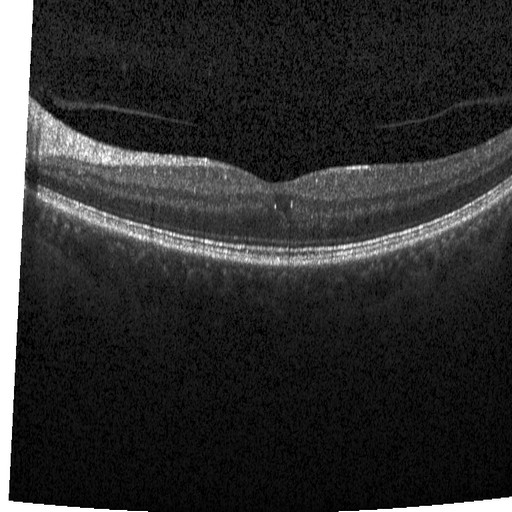
Macular OCT demonstrating diabetic macular edema (DME).